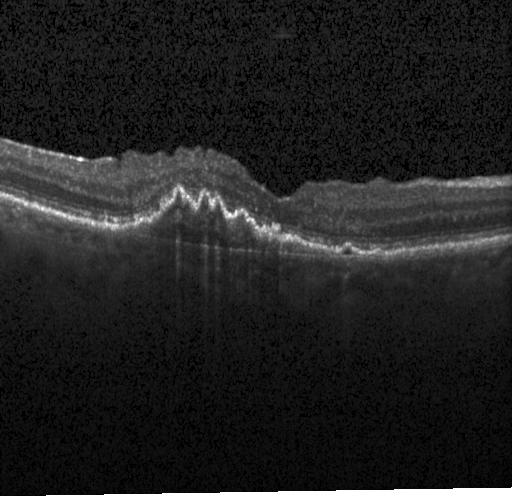 The scan shows choroidal neovascularization (CNV).